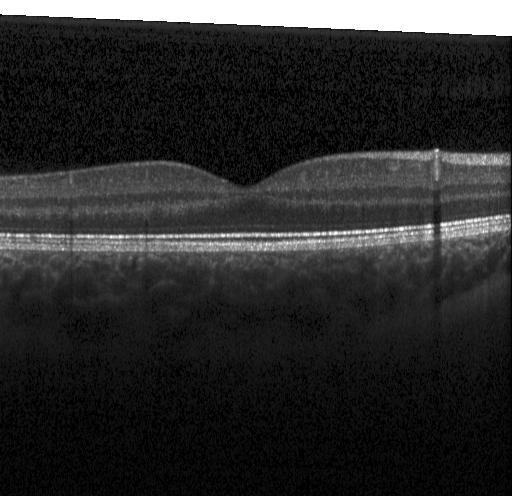 Retinal OCT cross-section, SD-OCT — Diagnosis: no CNV, DME, or drusen.